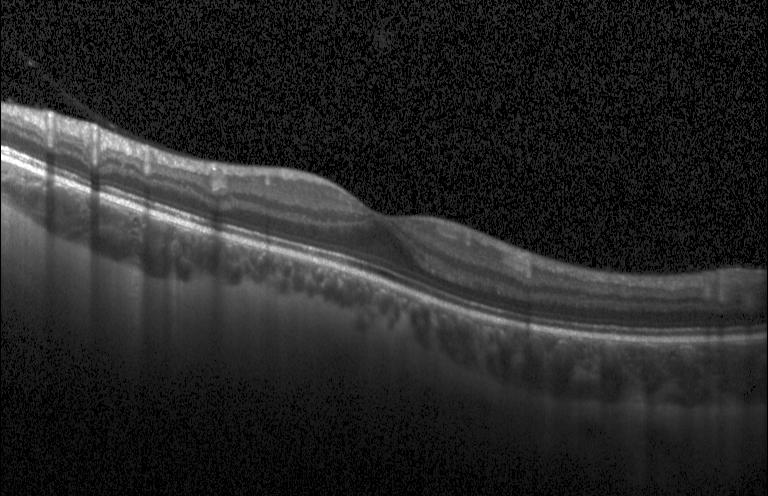
Dx: no CNV, DME, or drusen.